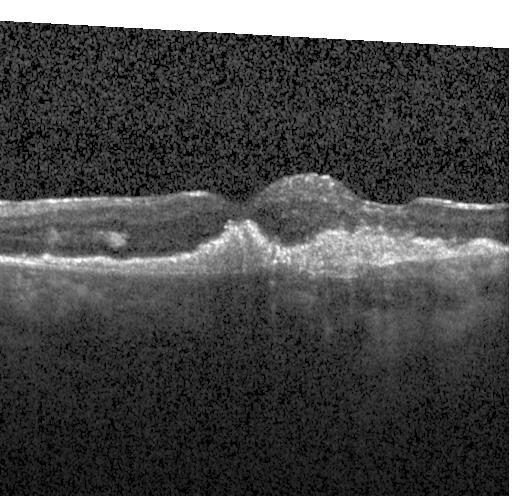

Spectral-domain optical coherence tomography · Heidelberg Spectralis · OCT line scan · macular scan.
Impression: a choroidal neovascular membrane.